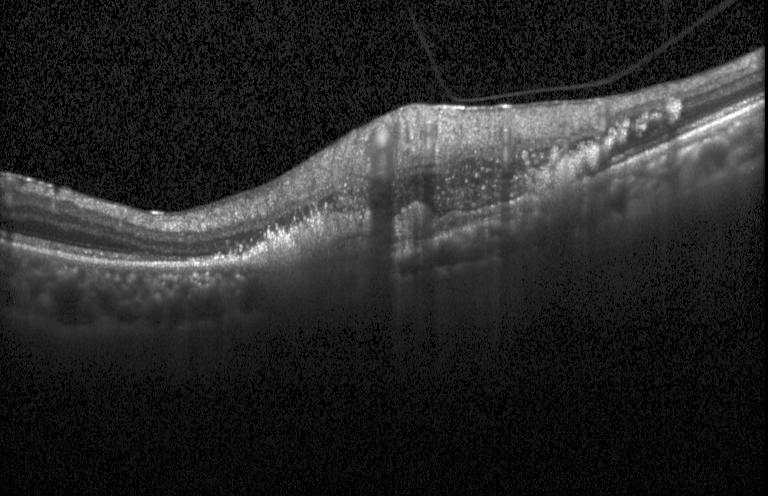
SD-OCT; through the macula; acquired on a Heidelberg Spectralis; OCT B-scan. This B-scan demonstrates CNV.